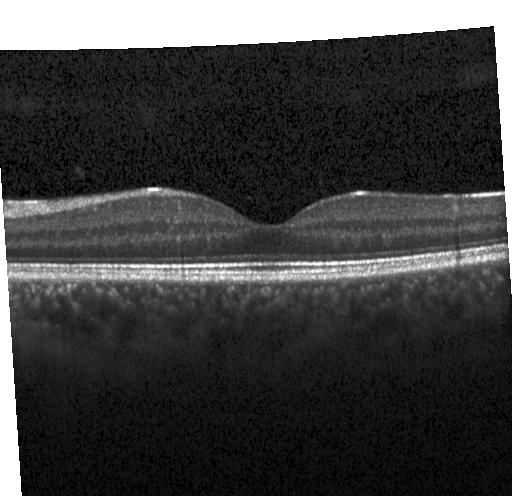 No choroidal neovascularization, diabetic macular edema, or drusen.